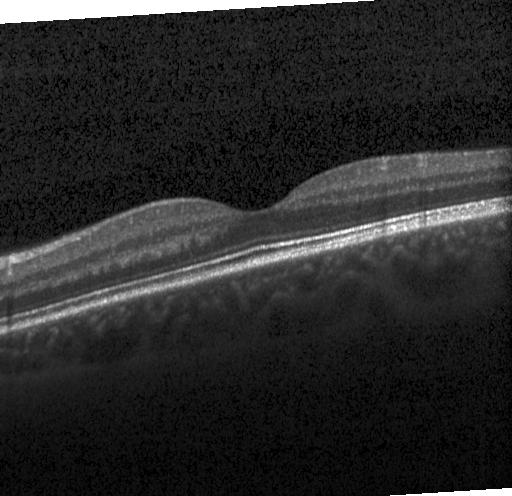

Optical coherence tomography scan
Dx: neither choroidal neovascularization, diabetic macular edema, nor drusen.